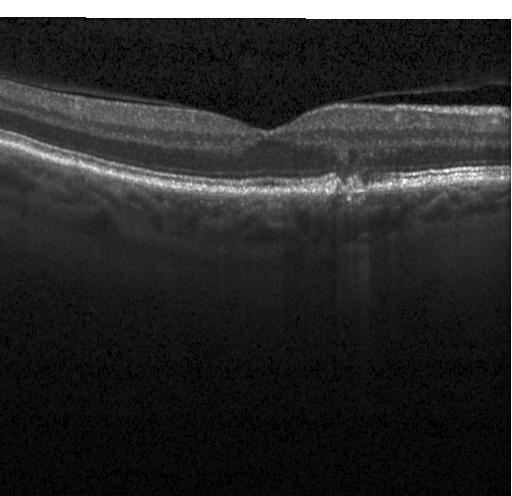 Retinal OCT cross-section showing drusen.